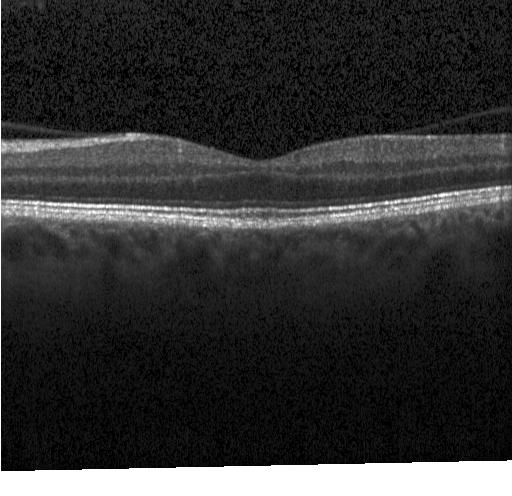
OCT B-scan showing no evidence of CNV, DME, or drusen.